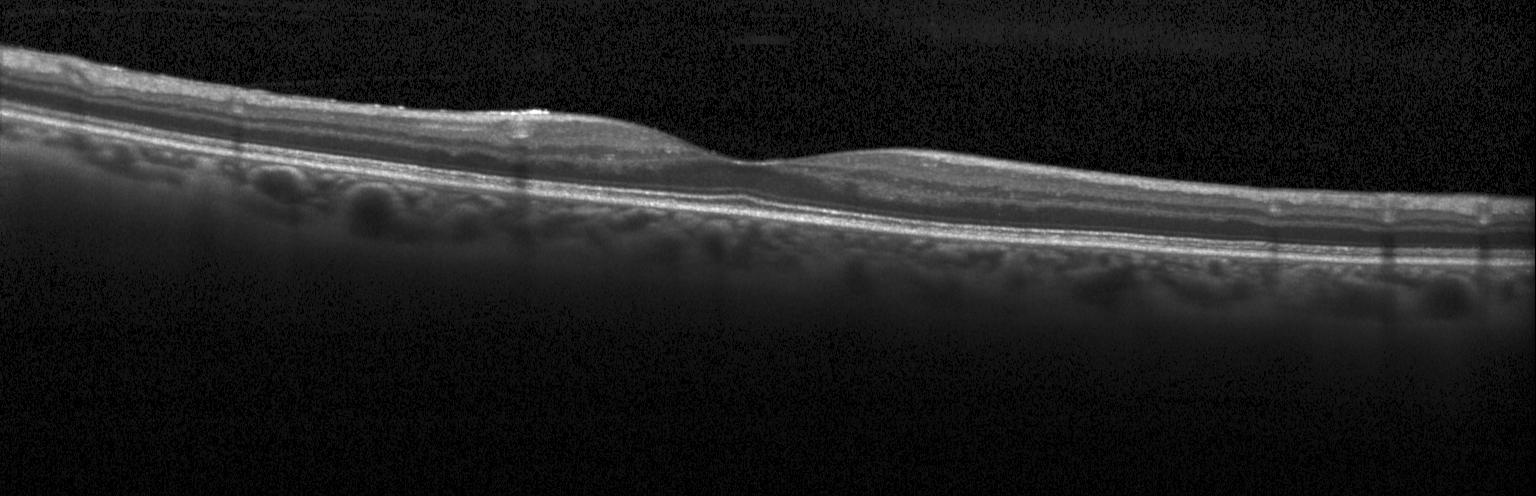
Optical coherence tomography B-scan. Impression: no choroidal neovascularization, diabetic macular edema, or drusen.